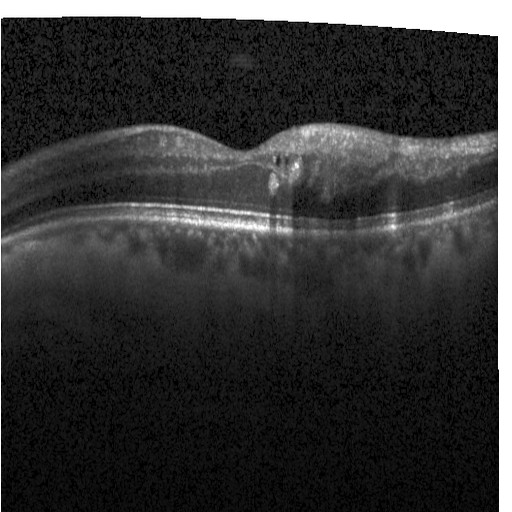
Diagnosis: diabetic macular edema.